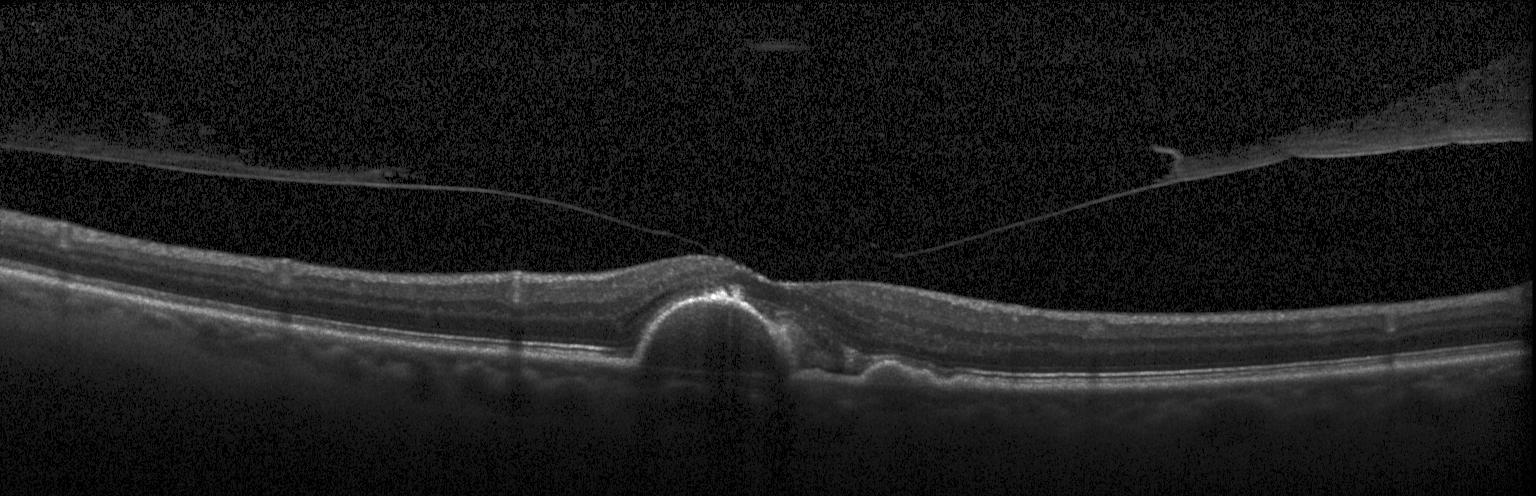
Optical coherence tomography B-scan. The scan shows a choroidal neovascular membrane.